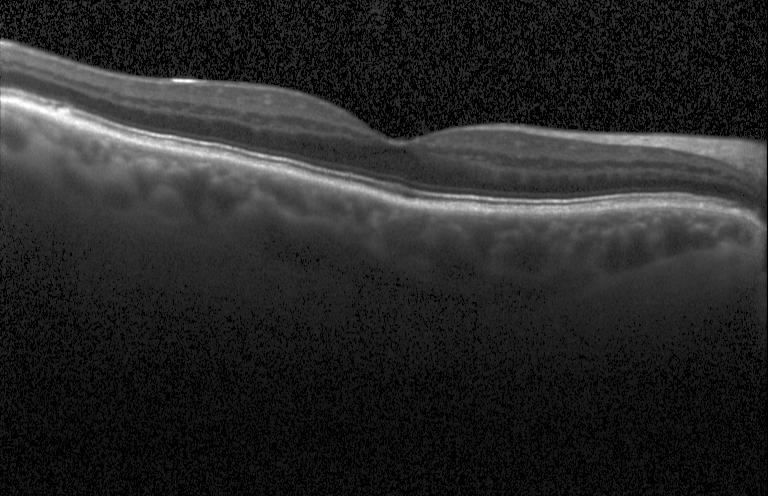 Diagnosis: no choroidal neovascularization, diabetic macular edema, or drusen.